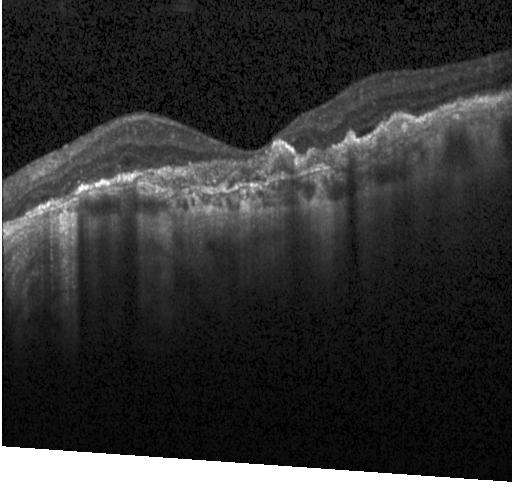
Choroidal neovascularization.